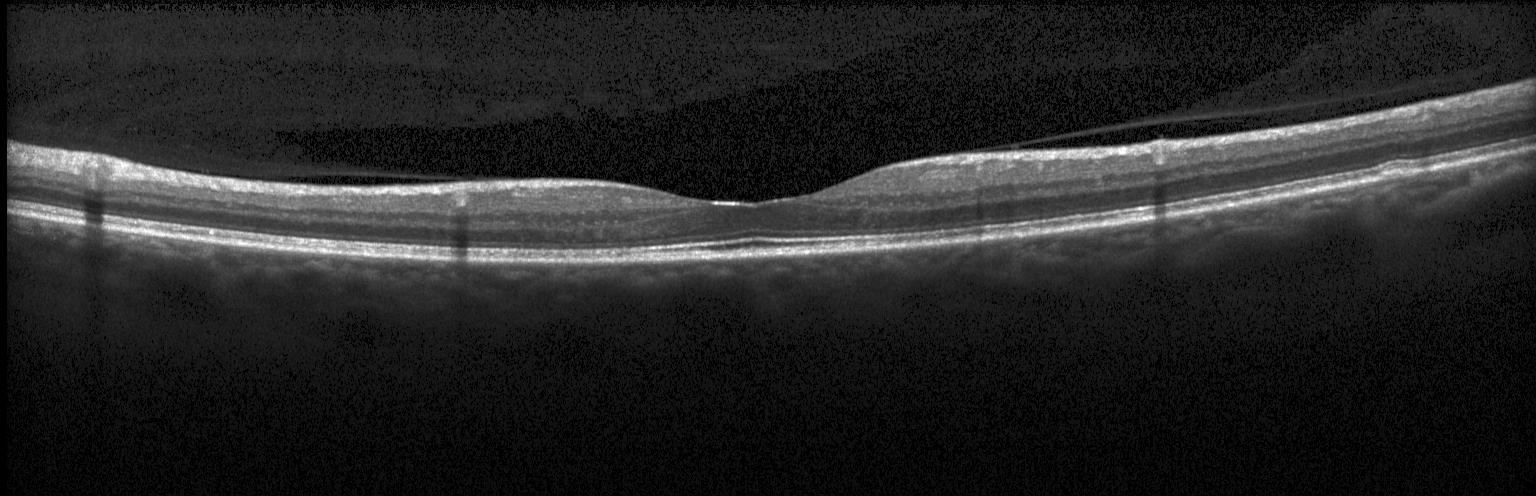

Heidelberg Spectralis OCT system. Optical coherence tomography B-scan — Finding: no CNV, DME, or drusen.